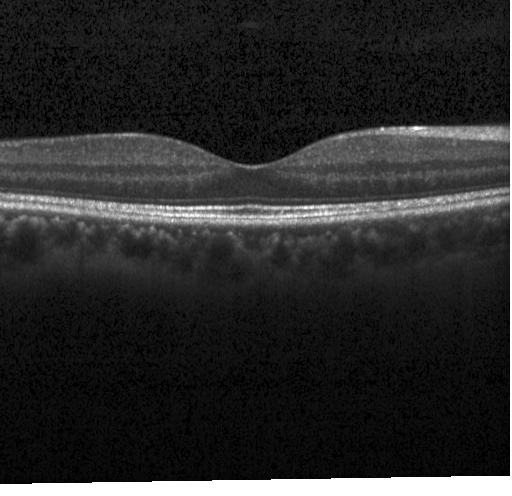 Retinal OCT cross-section, fovea-centered — Assessment: no evidence of choroidal neovascularization, diabetic macular edema, or drusen.